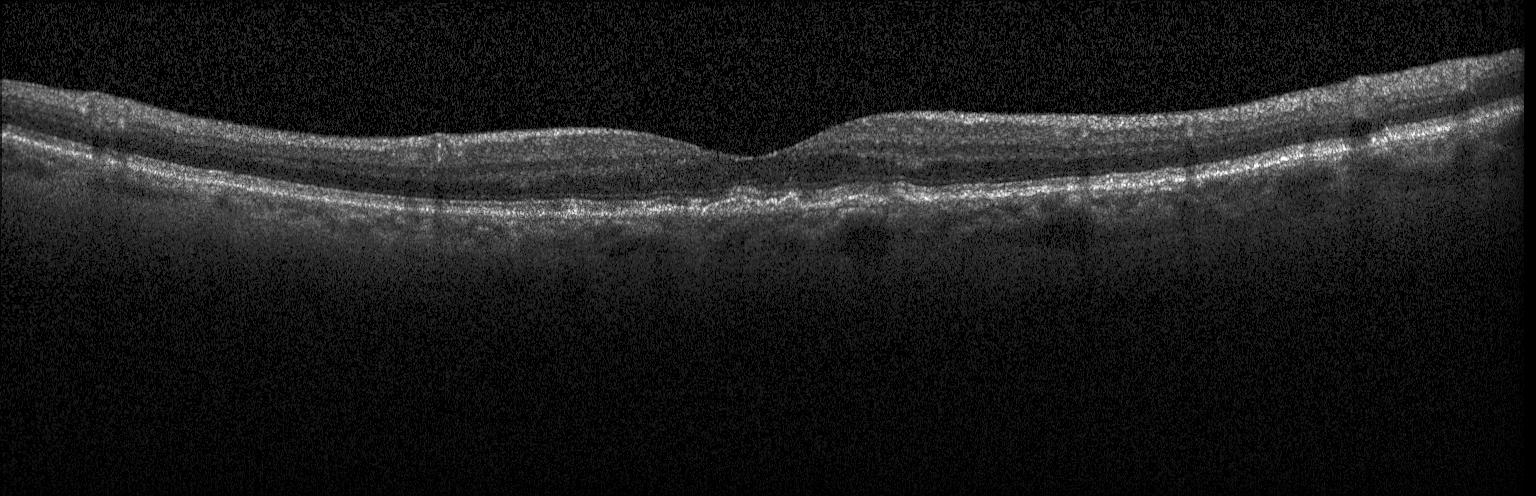 Horizontal scan through the fovea · SD-OCT · instrument: Heidelberg Spectralis · OCT line scan — Assessment: sub-RPE drusenoid deposits.